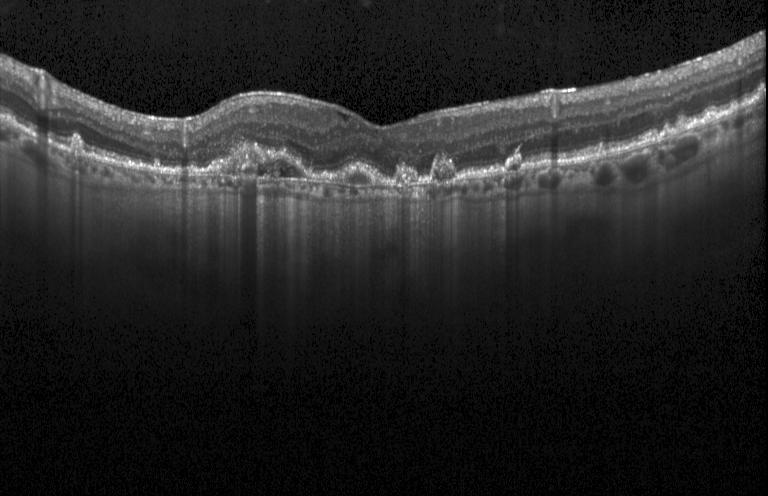

Optical coherence tomography scan
Impression: a choroidal neovascular membrane.